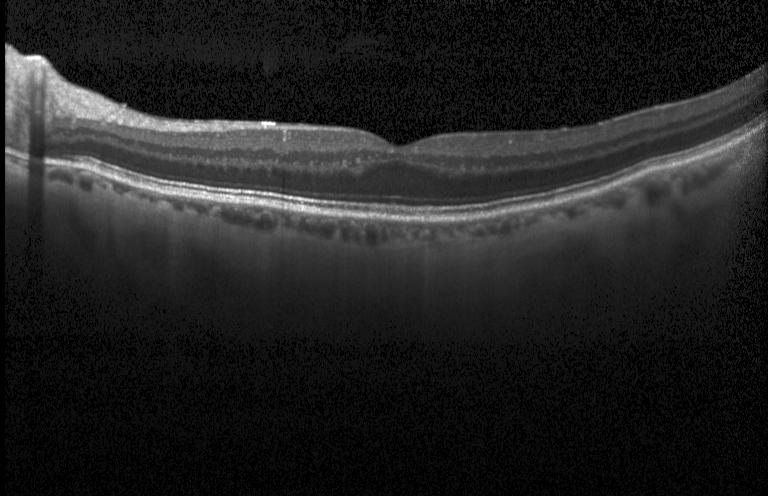
OCT line scan.
The scan shows no evidence of choroidal neovascularization, diabetic macular edema, or drusen.